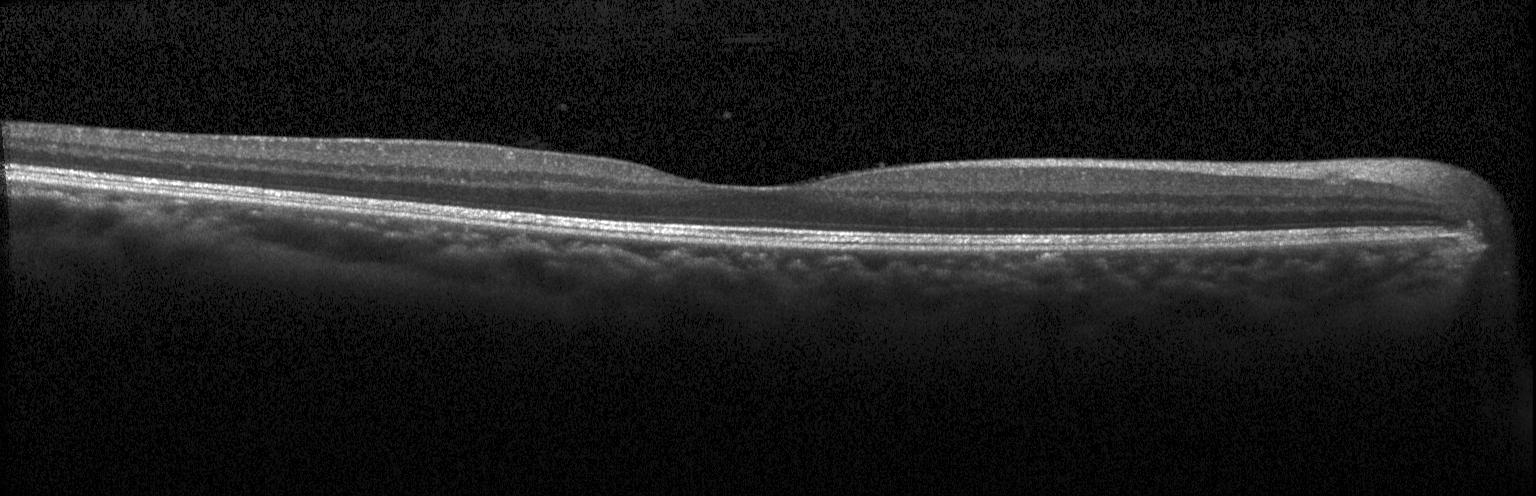
Horizontal scan through the fovea; spectral-domain optical coherence tomography; OCT B-scan; acquired on a Heidelberg Spectralis
Diagnosis: neither choroidal neovascularization, diabetic macular edema, nor drusen.